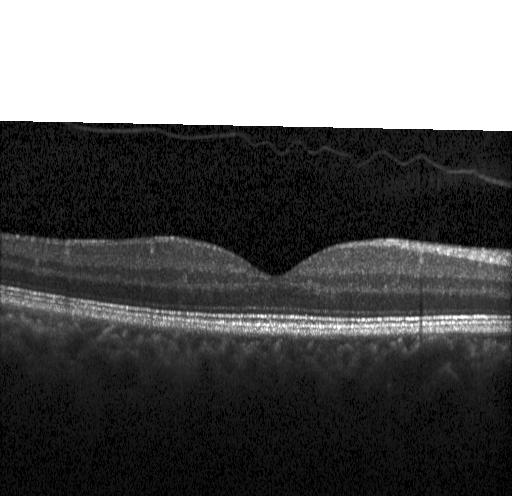

Macular scan, optical coherence tomography B-scan. No evidence of CNV, DME, or drusen.